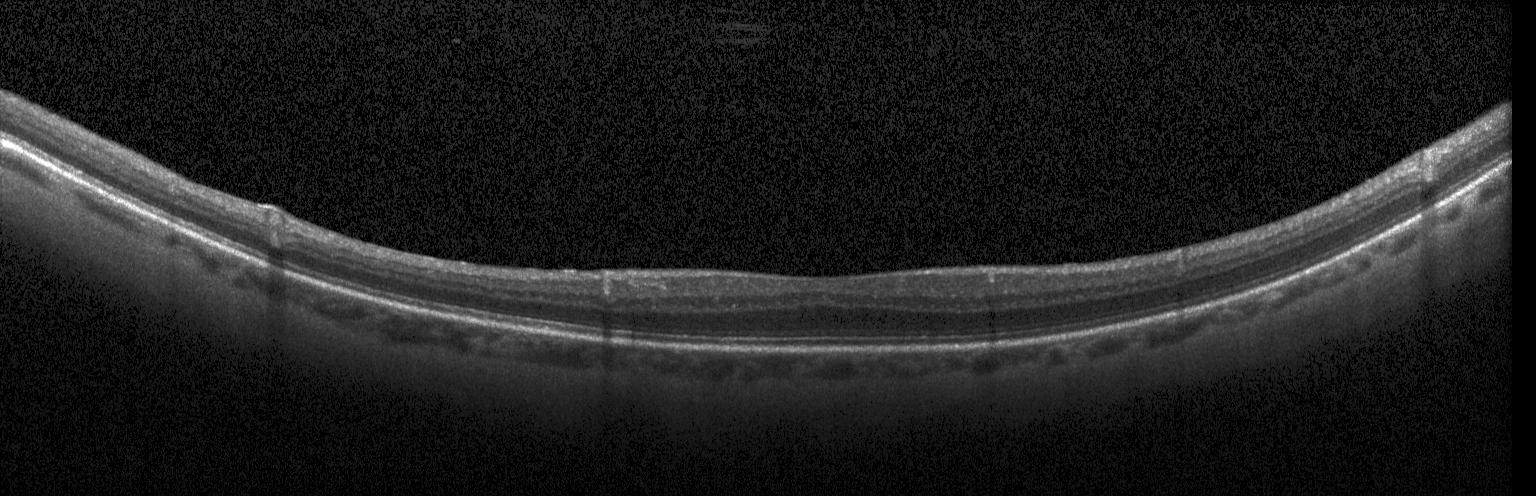
OCT B-scan showing no choroidal neovascularization, diabetic macular edema, or drusen.